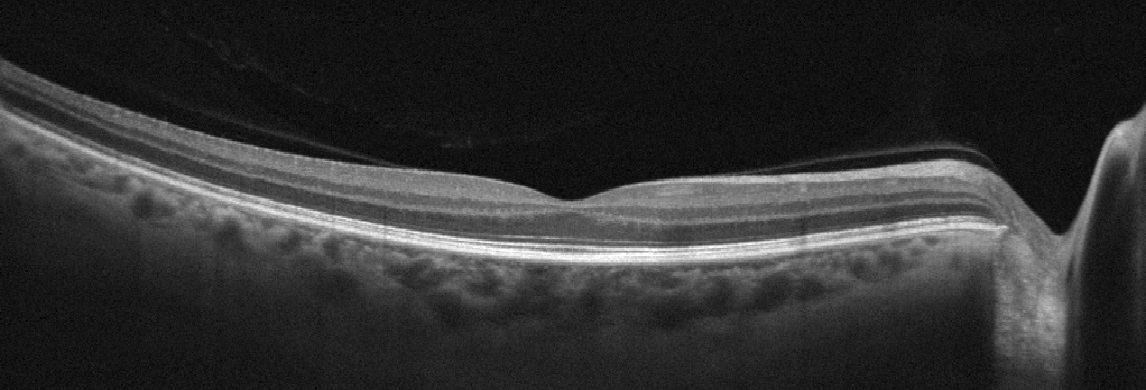
OCT B-scan showing no evidence of AMD, DME, ERM, RAO, RVO, or VID.